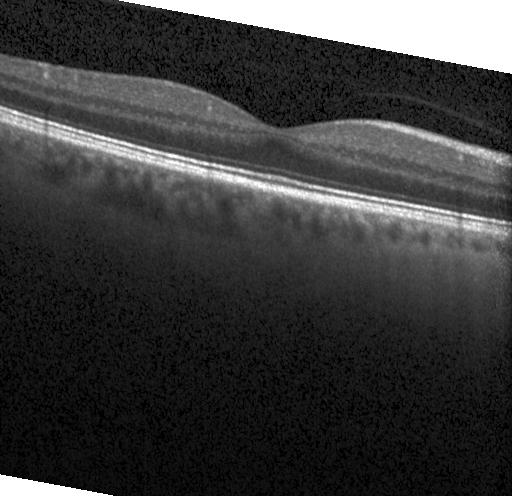

Diagnosis: neither choroidal neovascularization, diabetic macular edema, nor drusen.